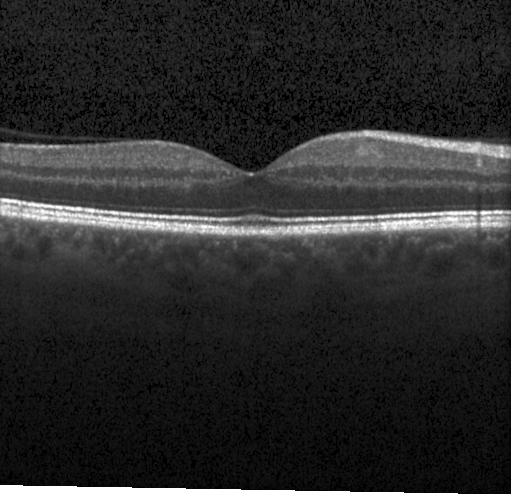
Optical coherence tomography scan · SD-OCT · macular scan · Heidelberg Spectralis OCT system
Impression: neither CNV, DME, nor drusen.